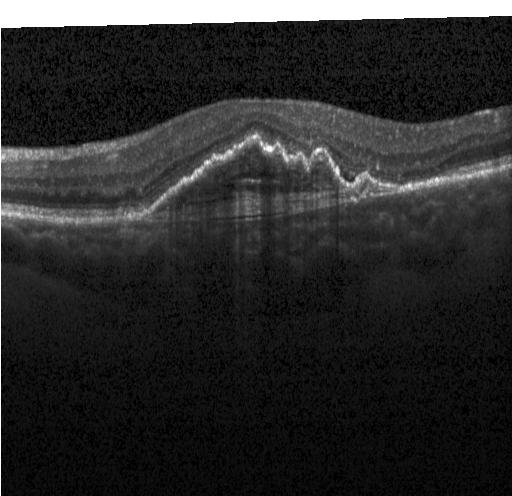

Optical coherence tomography scan — Impression: choroidal neovascularization.